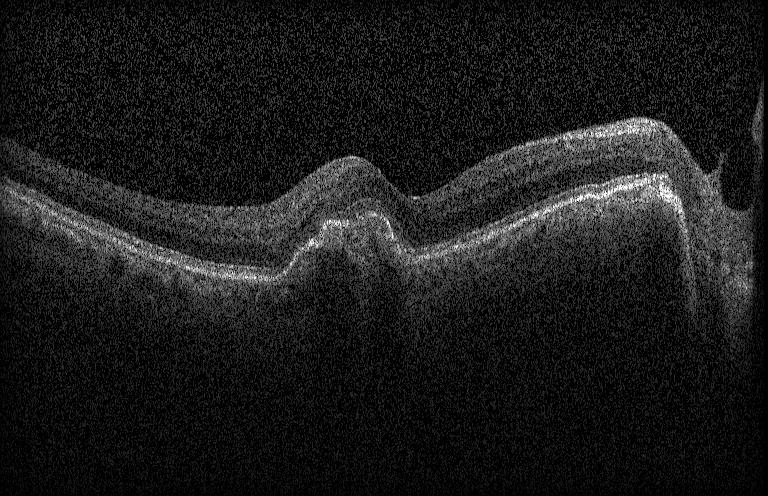 Impression: CNV.